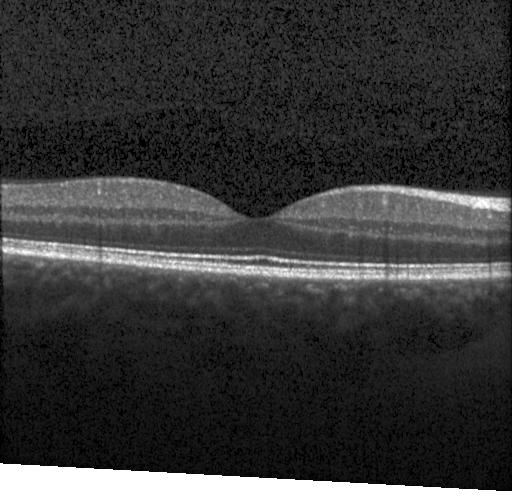 Instrument: Heidelberg Spectralis. Spectral-domain OCT. Retinal OCT B-scan. Fovea-centered — Finding: no choroidal neovascularization, no diabetic macular edema, and no drusen.